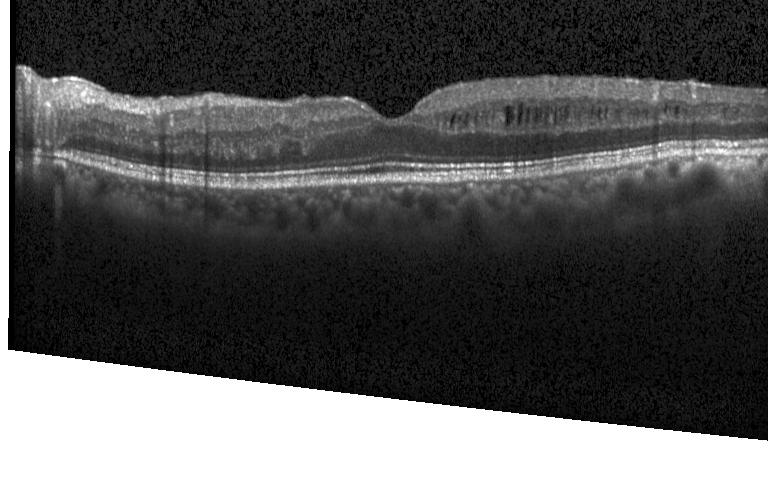

Heidelberg Spectralis · optical coherence tomography scan.
Dx: DME.